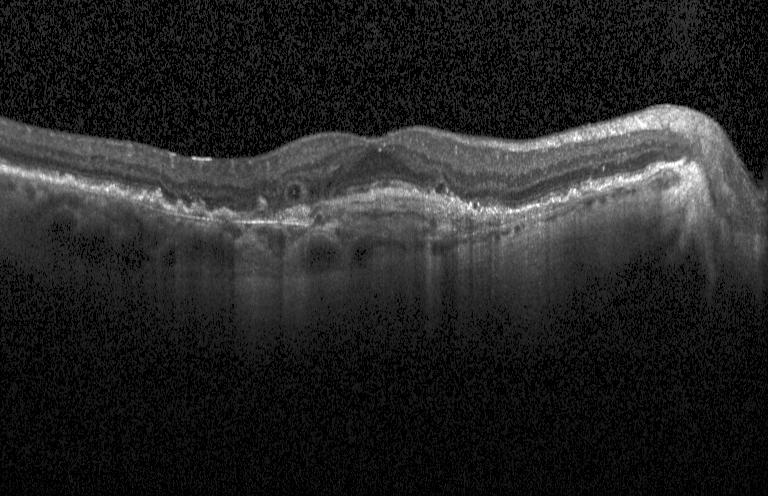
Retinal OCT B-scan.
Assessment: a choroidal neovascular membrane.